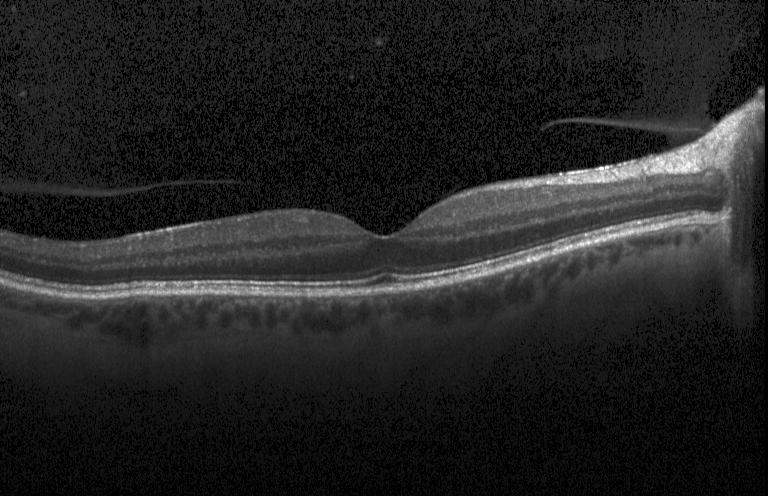 Through the macula. SD-OCT. Optical coherence tomography scan.
Macular OCT: neither choroidal neovascularization, diabetic macular edema, nor drusen.